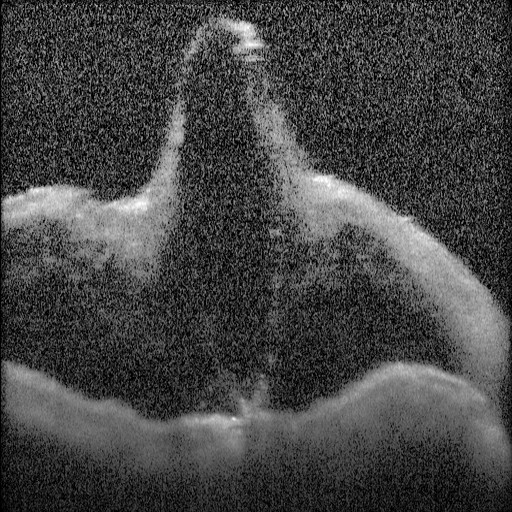 OCT finding: diabetic macular edema.